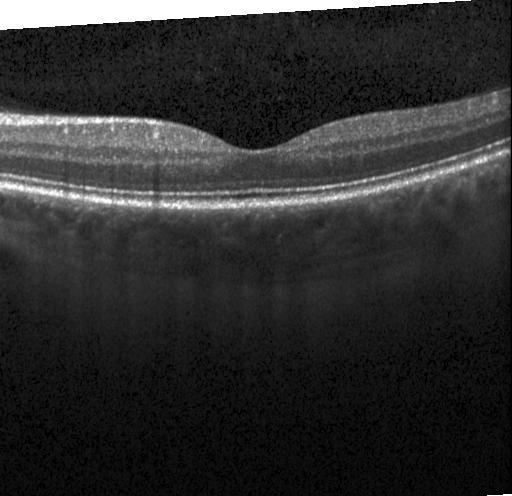 OCT B-scan showing no evidence of CNV, DME, or drusen.